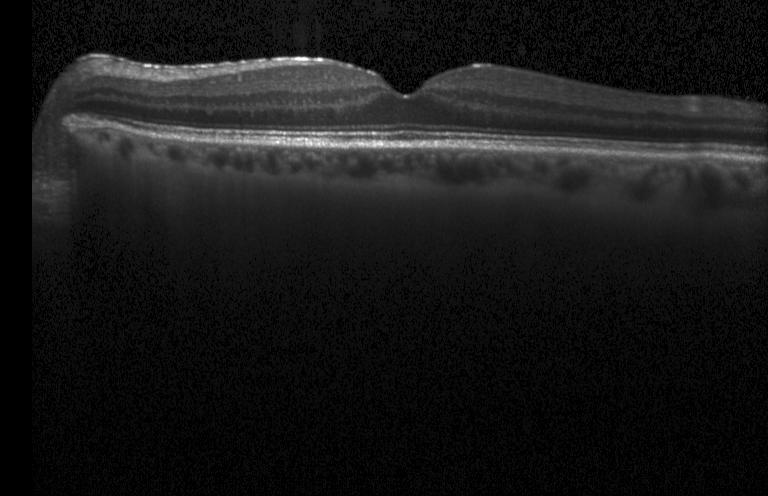
SD-OCT. Through the macula. Acquired on a Heidelberg Spectralis. OCT B-scan.
Macular OCT: no choroidal neovascularization, diabetic macular edema, or drusen.